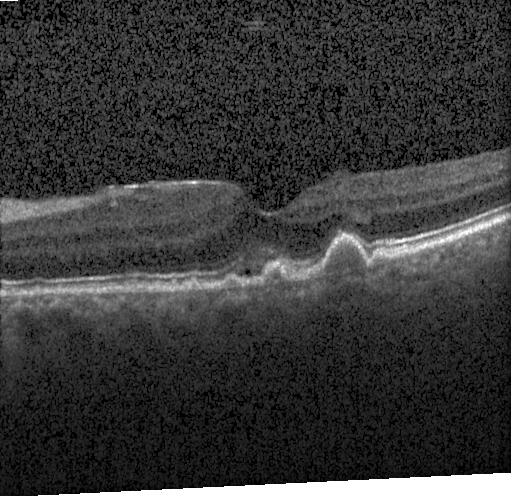

This B-scan demonstrates drusen.